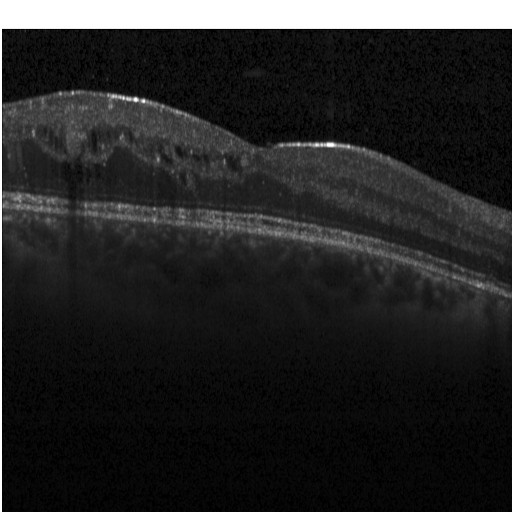

Assessment: diabetic macular edema (DME).